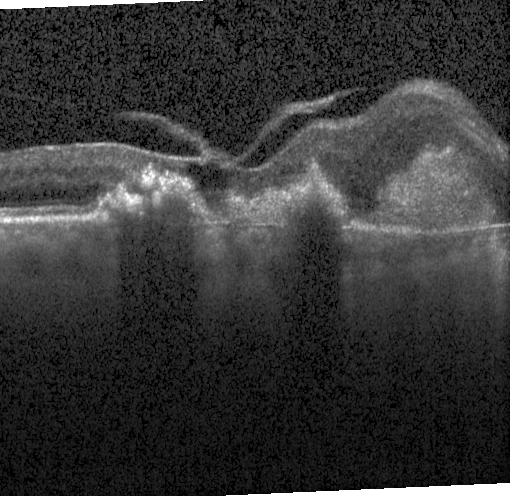
Dx: a choroidal neovascular membrane.